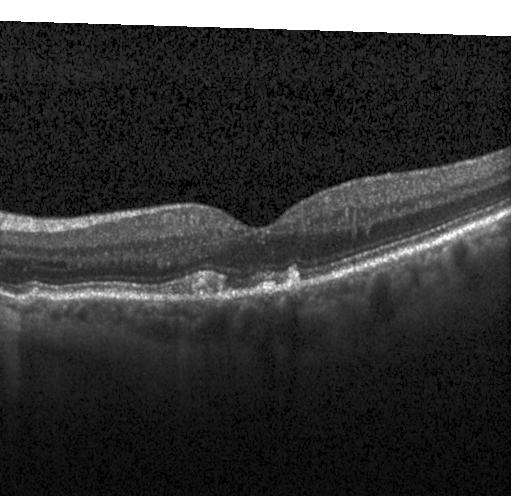

Optical coherence tomography B-scan, SD-OCT, Heidelberg Spectralis, macular scan
Macular OCT: drusen.